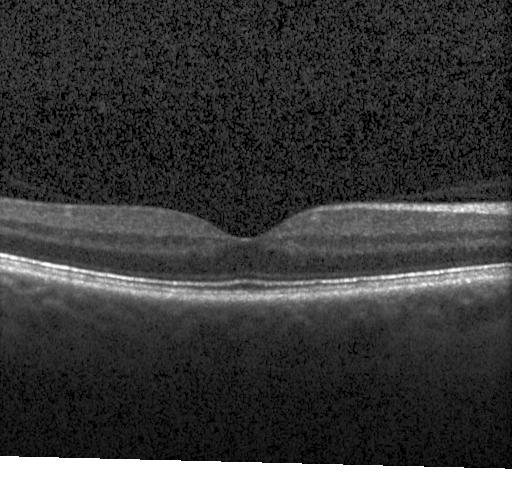 Macular OCT demonstrating no CNV, DME, or drusen.